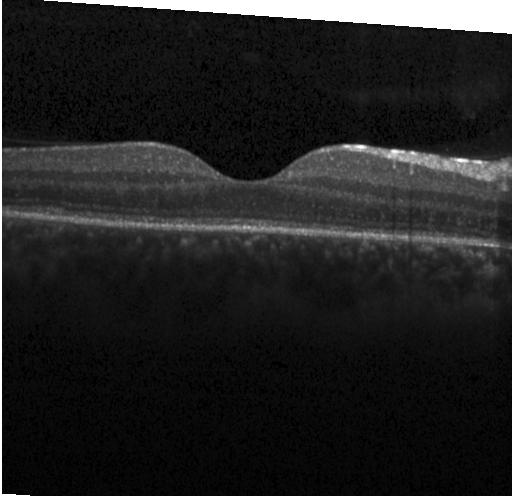
Optical coherence tomography B-scan, Heidelberg Spectralis OCT system, spectral-domain OCT, macular scan
Diagnosis: no choroidal neovascularization, diabetic macular edema, or drusen.